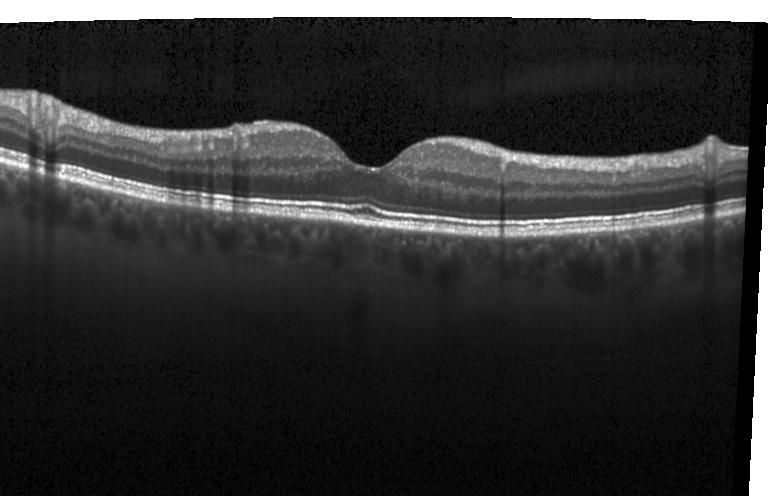 Macular OCT demonstrating no evidence of CNV, DME, or drusen.